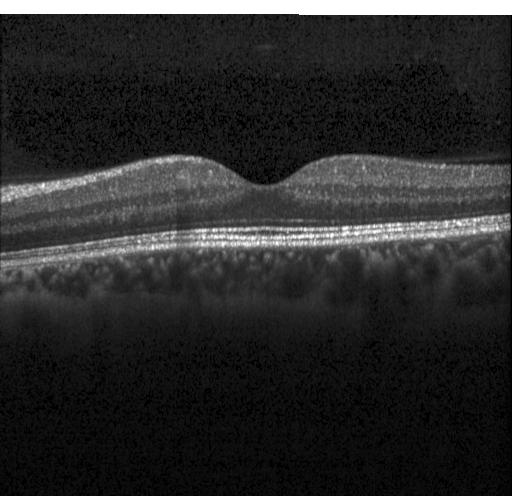

OCT B-scan showing no CNV, DME, or drusen.